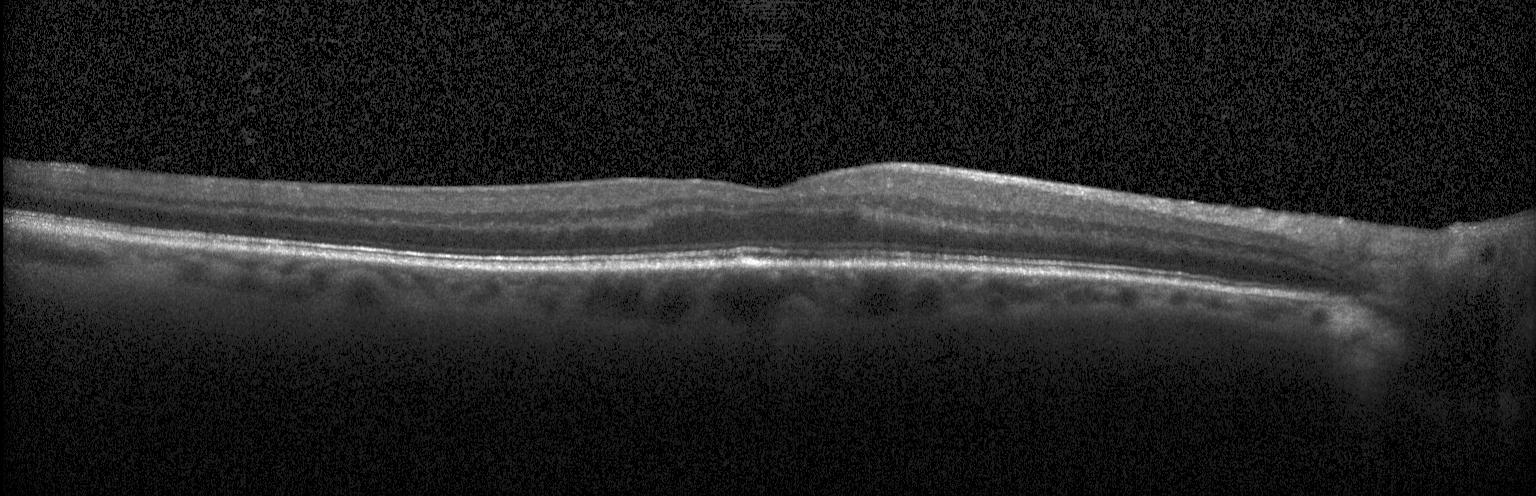
Neither choroidal neovascularization, diabetic macular edema, nor drusen.